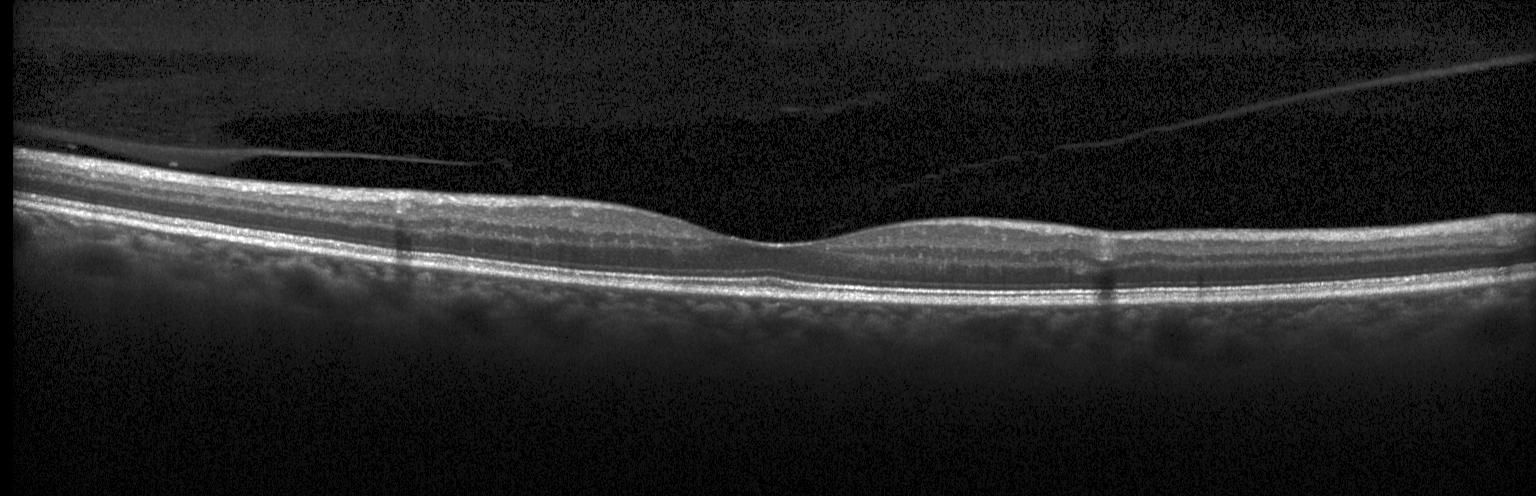 Diagnosis: no evidence of choroidal neovascularization, diabetic macular edema, or drusen.